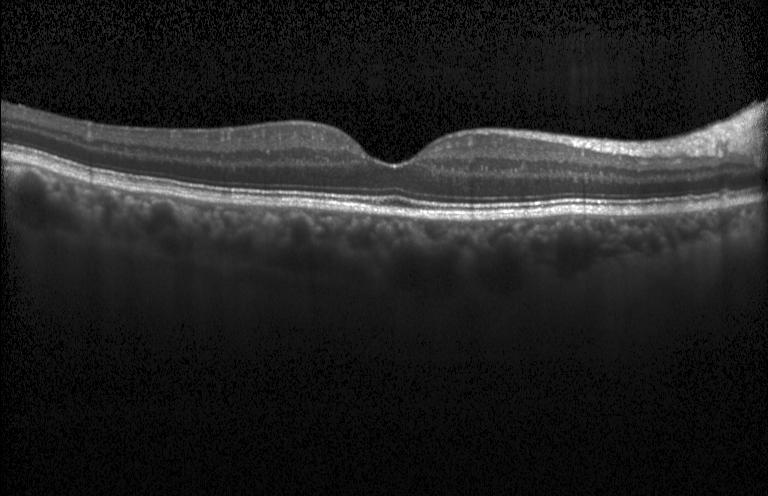

OCT B-scan. Heidelberg Spectralis OCT system. Fovea-centered. SD-OCT — Assessment: no CNV, DME, or drusen.